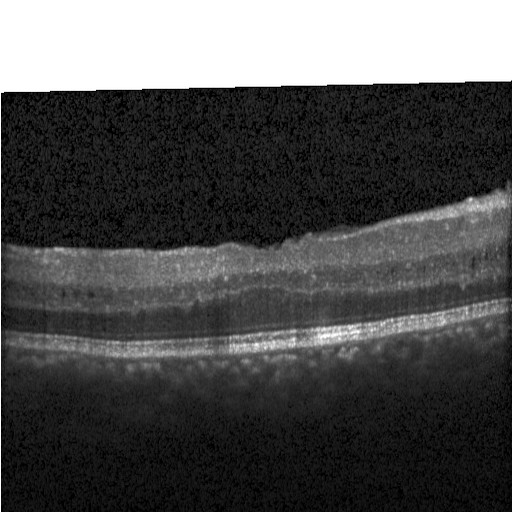

Macular scan; retinal OCT cross-section.
Diagnosis: diabetic macular edema.